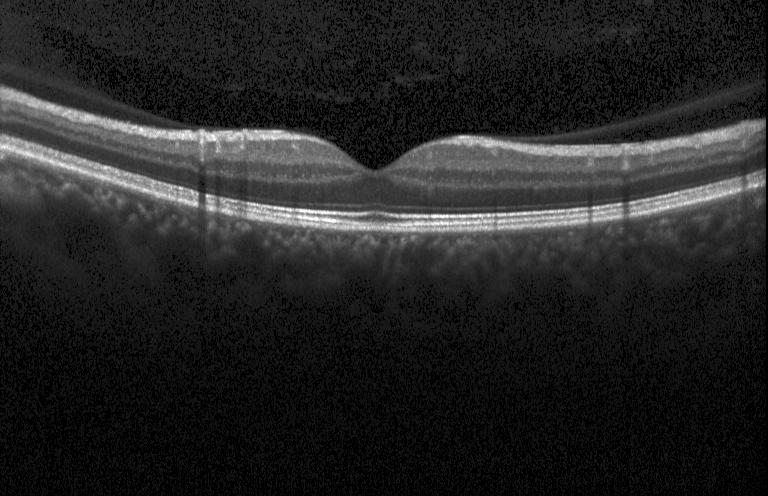

Dx: no evidence of choroidal neovascularization, diabetic macular edema, or drusen.